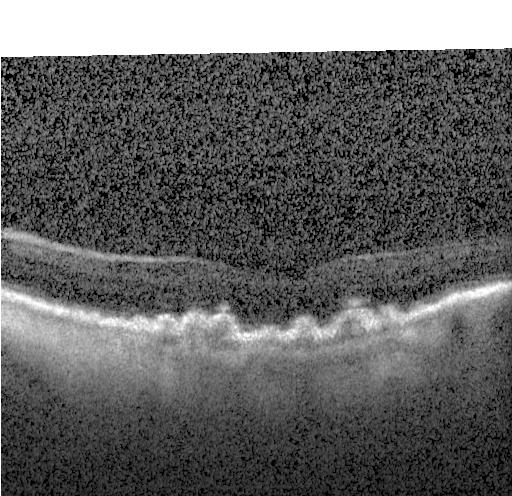 Macular OCT demonstrating multiple drusen.